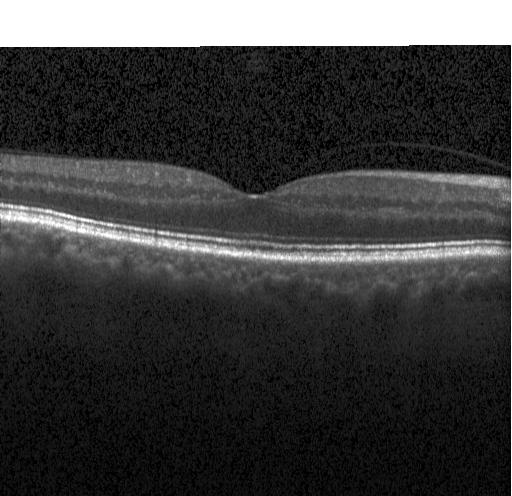 Retinal OCT cross-section · spectral-domain optical coherence tomography · through the macula — Assessment: no choroidal neovascularization, no diabetic macular edema, and no drusen.